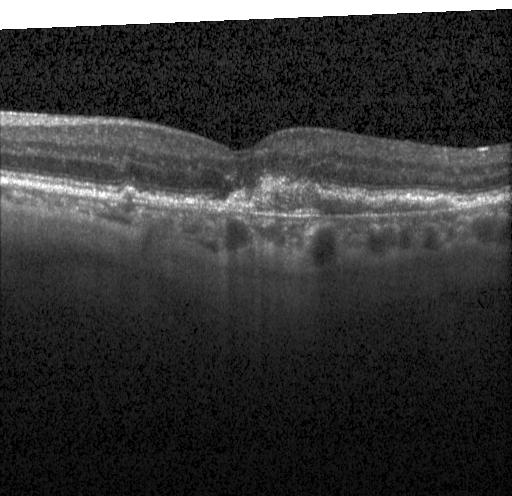

Retinal OCT B-scan.
A choroidal neovascular membrane.